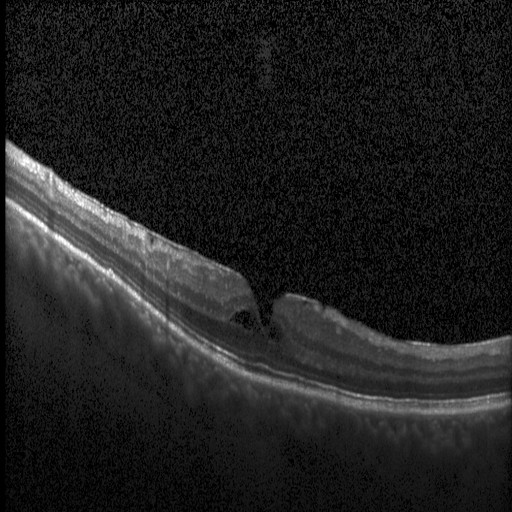
Instrument: Heidelberg Spectralis. SD-OCT. OCT line scan.
Macular OCT: diabetic macular edema (DME).